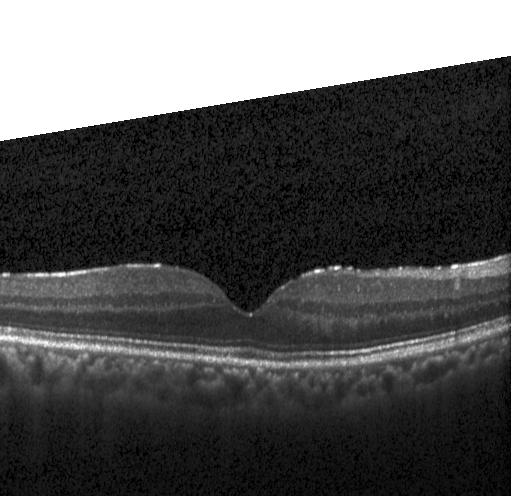

Acquired on a Heidelberg Spectralis · retinal OCT cross-section · macular scan.
Dx: no CNV, no DME, and no drusen.